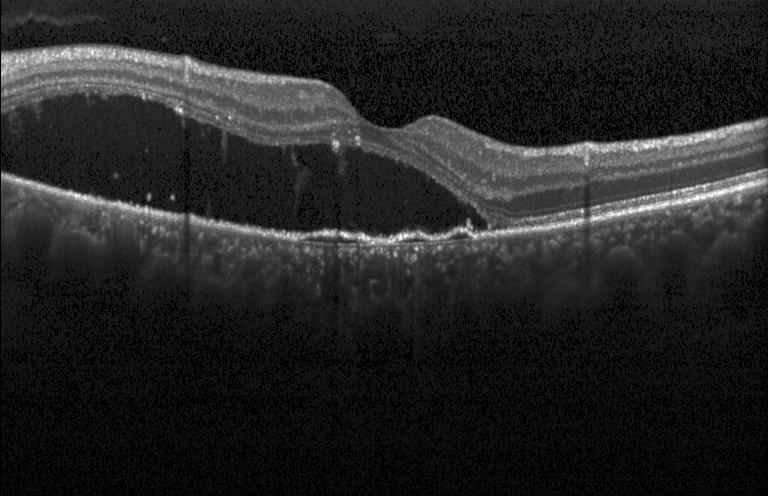 Finding: a choroidal neovascular membrane.